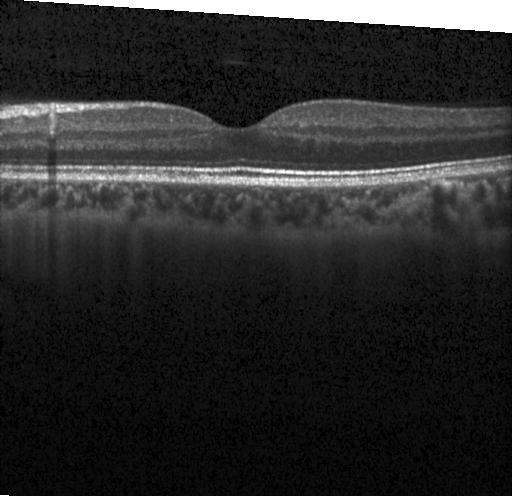
Macular OCT demonstrating no CNV, DME, or drusen.